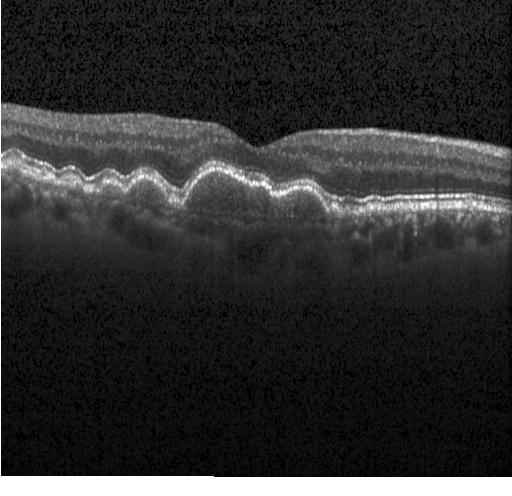
SD-OCT · instrument: Heidelberg Spectralis · macular scan · OCT line scan
Finding: drusen.